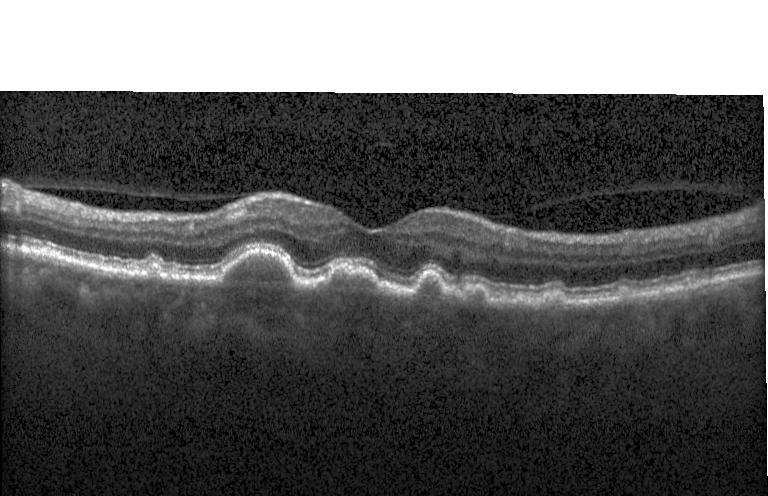

OCT B-scan. Centered on the fovea. Heidelberg Spectralis OCT system
The scan shows sub-RPE drusenoid deposits.